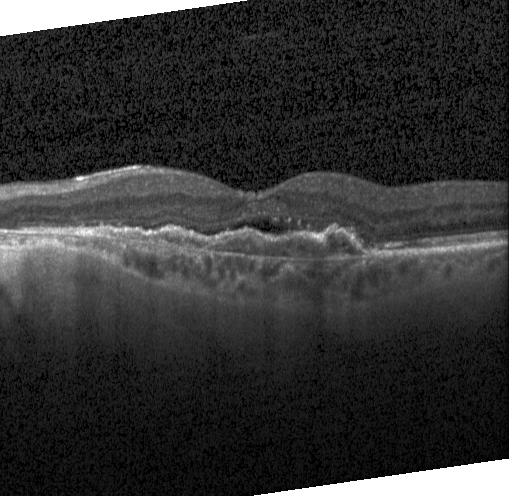 OCT finding: CNV.